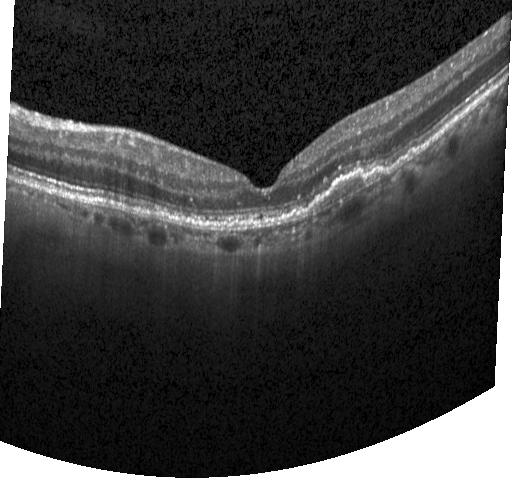 Heidelberg Spectralis · horizontal scan through the fovea · spectral-domain optical coherence tomography · optical coherence tomography scan — Impression: a choroidal neovascular membrane.